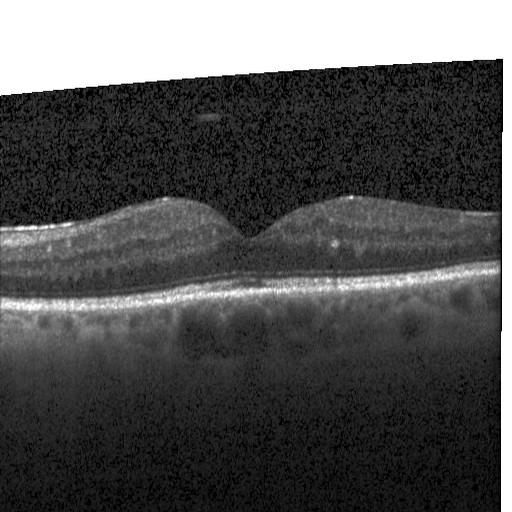

Retinal OCT cross-section; Heidelberg Spectralis; spectral-domain OCT.
The scan shows DME.